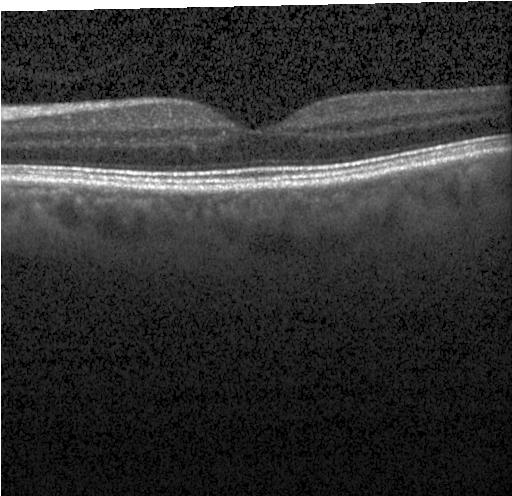 Retinal OCT cross-section. No choroidal neovascularization, no diabetic macular edema, and no drusen.